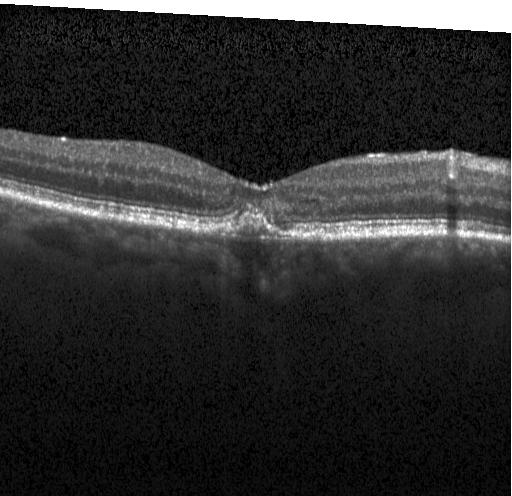

Acquired on a Heidelberg Spectralis; SD-OCT; centered on the fovea; OCT B-scan.
Diagnosis: a choroidal neovascular membrane.